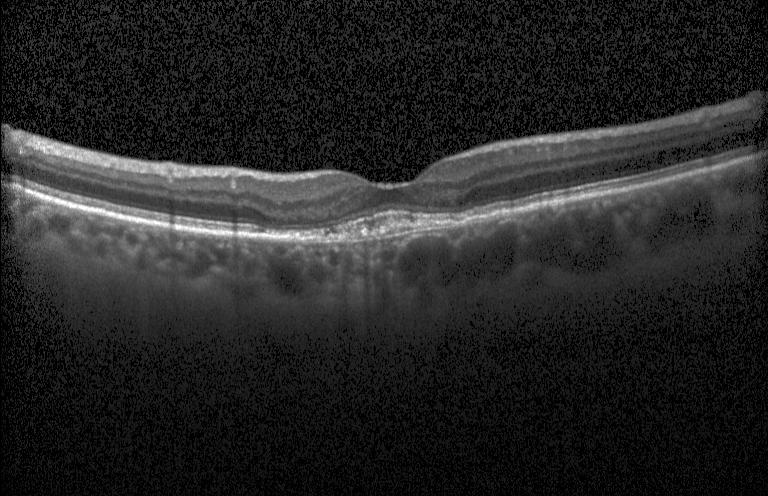
Impression: a choroidal neovascular membrane.